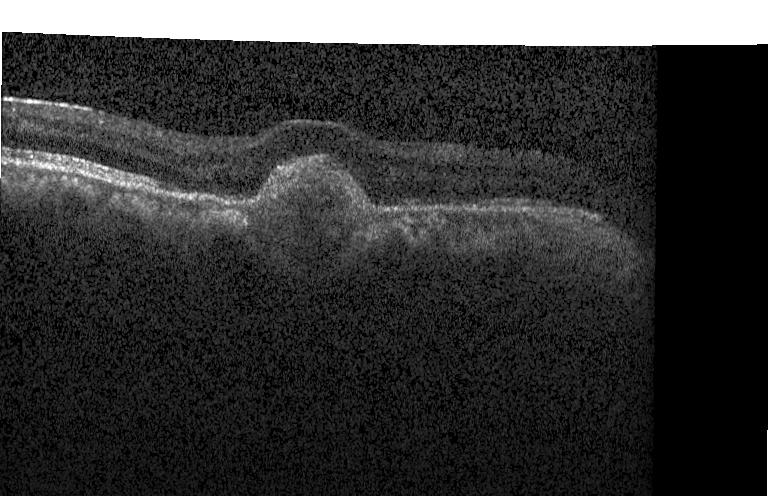 OCT B-scan · Heidelberg Spectralis · fovea-centered · spectral-domain optical coherence tomography.
Diagnosis: a choroidal neovascular membrane.